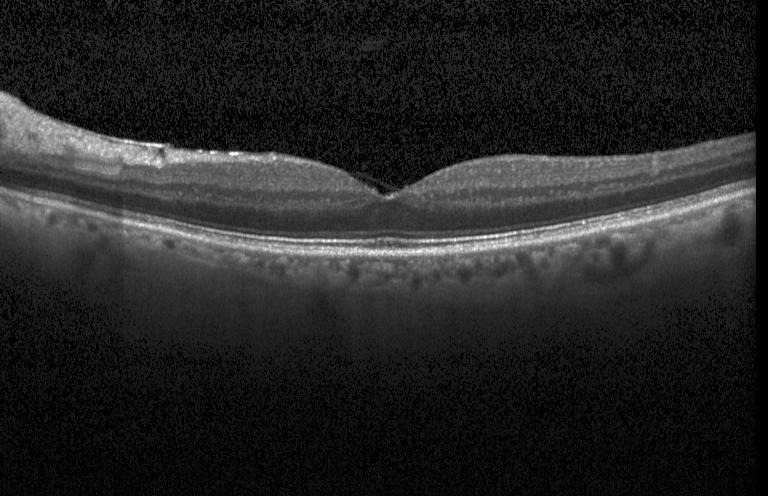

Impression: neither choroidal neovascularization, diabetic macular edema, nor drusen.